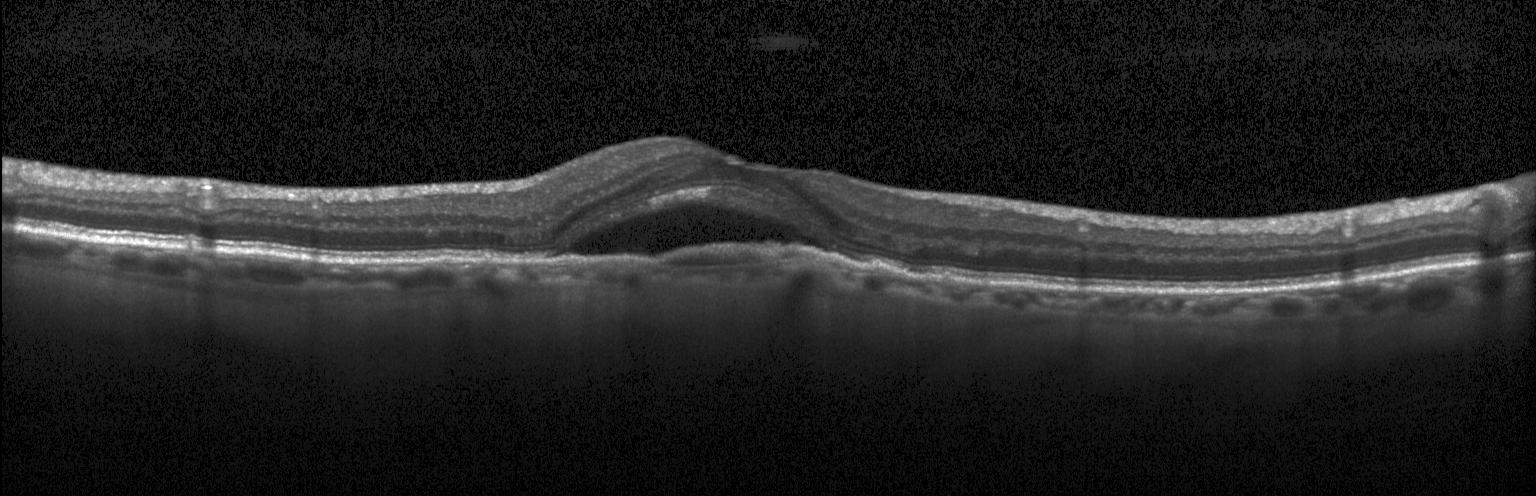

Optical coherence tomography scan. Centered on the fovea.
Finding: choroidal neovascularization (CNV).